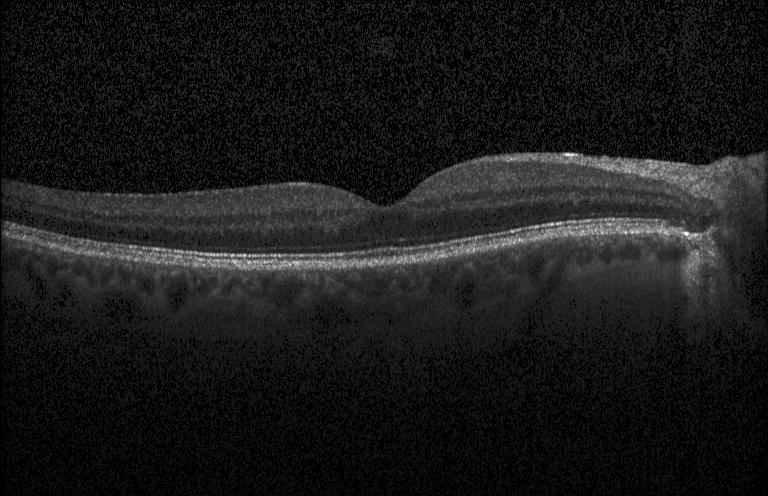

This B-scan demonstrates neither choroidal neovascularization, diabetic macular edema, nor drusen.